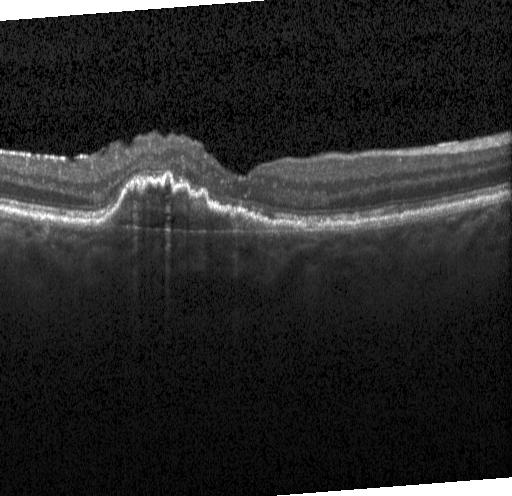 Dx: a choroidal neovascular membrane.